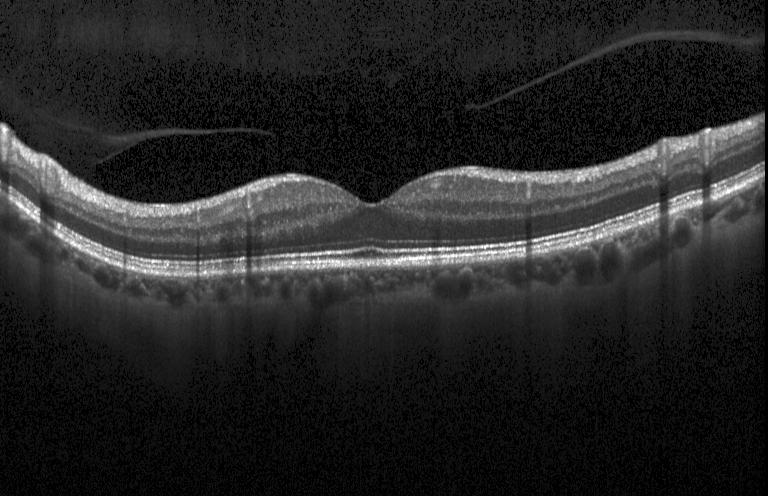
Retinal OCT B-scan.
The scan shows no choroidal neovascularization, no diabetic macular edema, and no drusen.